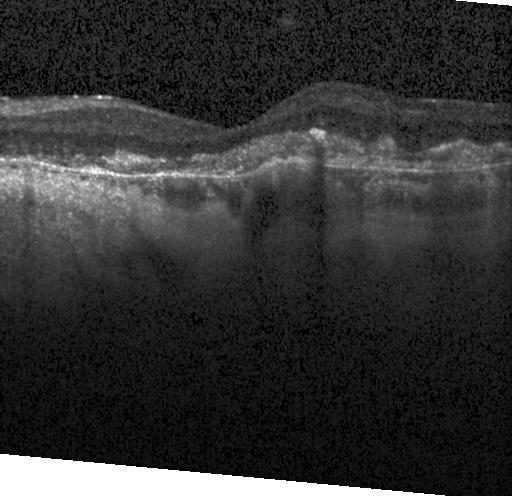 This B-scan demonstrates choroidal neovascularization (CNV).